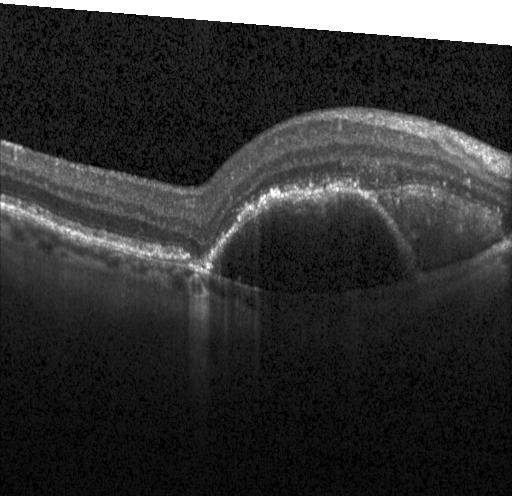
Spectral-domain OCT B-scan: a choroidal neovascular membrane.